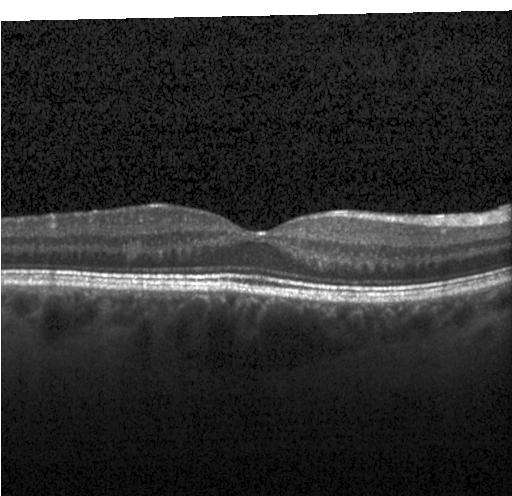

Centered on the fovea; retinal OCT cross-section.
No CNV, no DME, and no drusen.